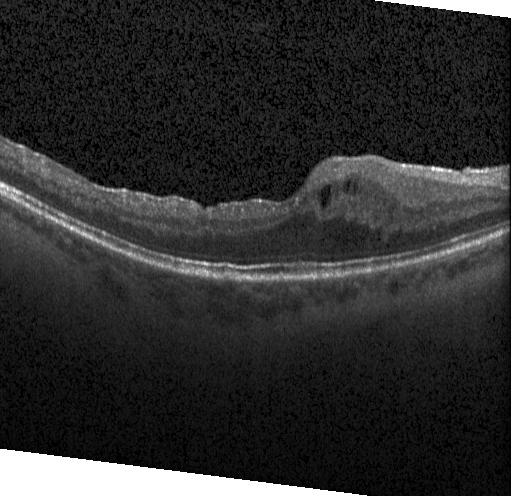 Diagnosis: diabetic macular edema (DME).